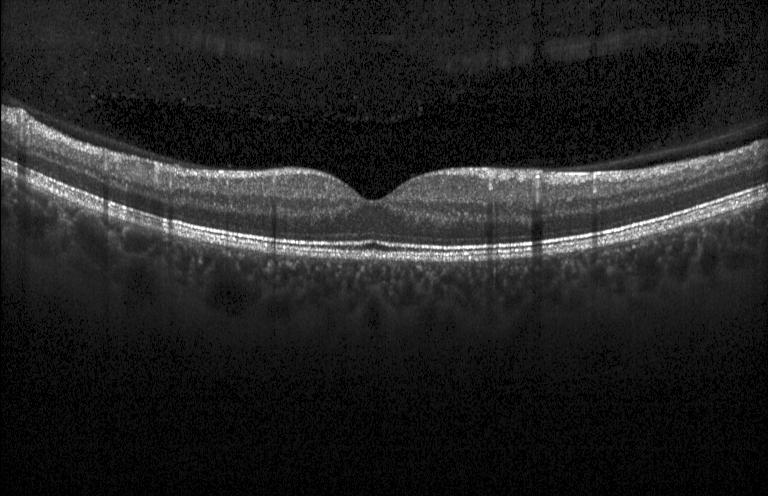

Spectral-domain OCT B-scan: no choroidal neovascularization, no diabetic macular edema, and no drusen.